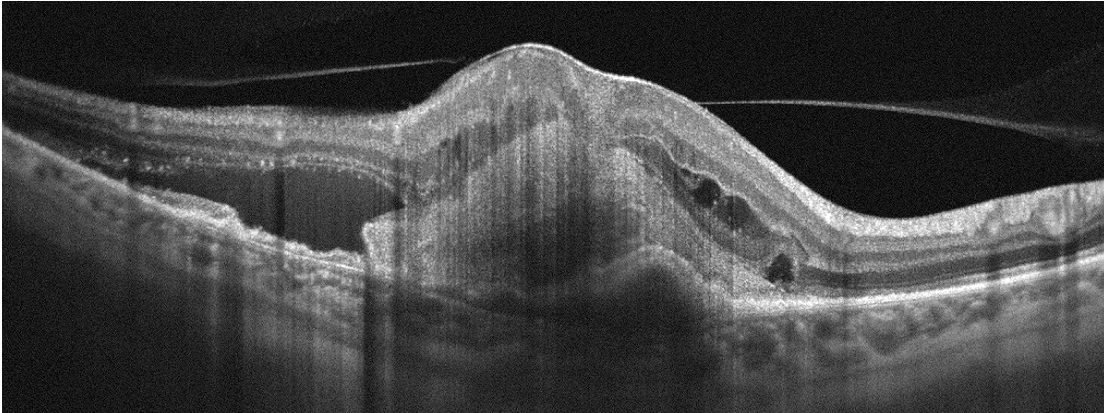
Retinal OCT cross-section · fovea-centered · Optovue Avanti RTVue XR.
Macular OCT: age-related macular degeneration (AMD).